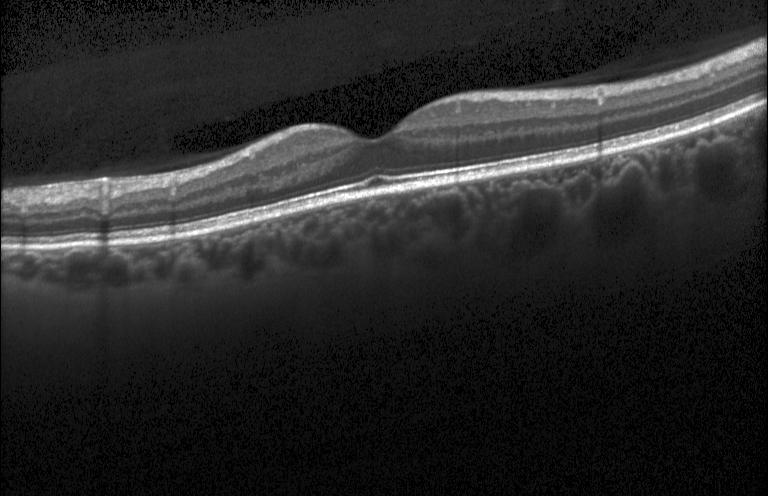
Retinal OCT B-scan. Heidelberg Spectralis. SD-OCT. Through the macula. Impression: neither CNV, DME, nor drusen.